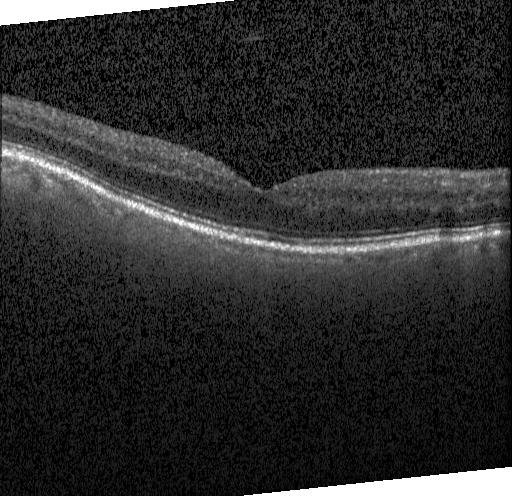 OCT line scan. This B-scan demonstrates no choroidal neovascularization, no diabetic macular edema, and no drusen.